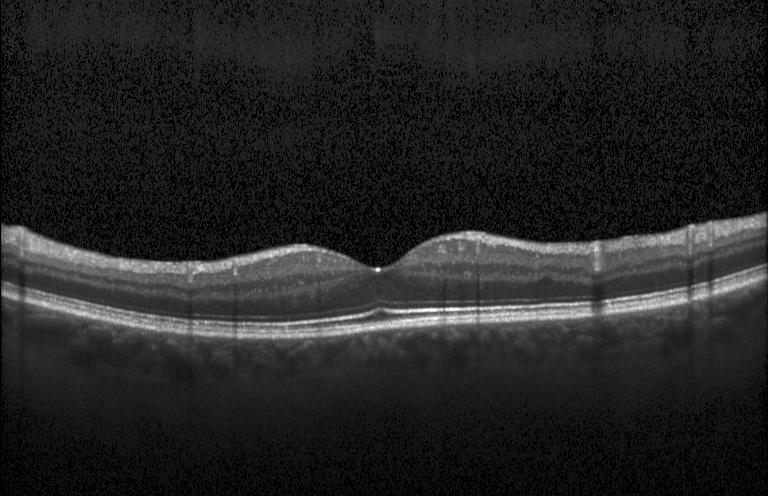 Spectral-domain optical coherence tomography, optical coherence tomography scan.
Diagnosis: no choroidal neovascularization, no diabetic macular edema, and no drusen.